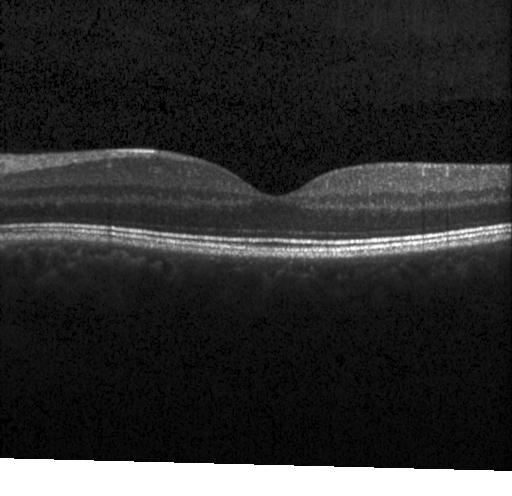 OCT B-scan — Finding: no choroidal neovascularization, diabetic macular edema, or drusen.